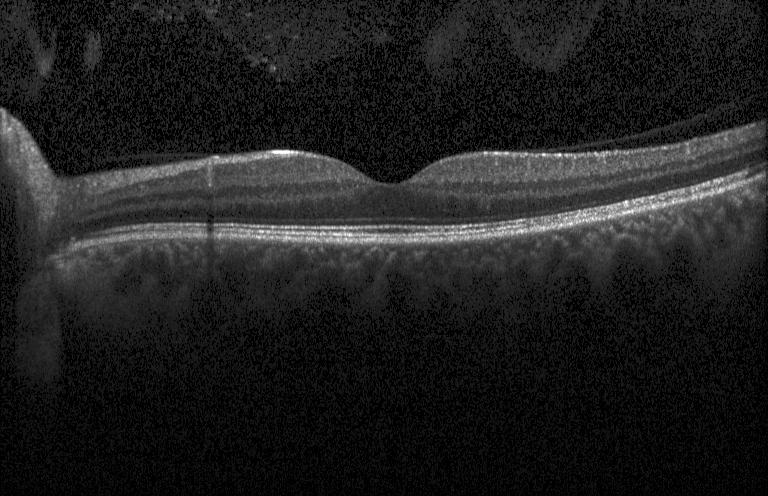 OCT finding: no choroidal neovascularization, diabetic macular edema, or drusen.